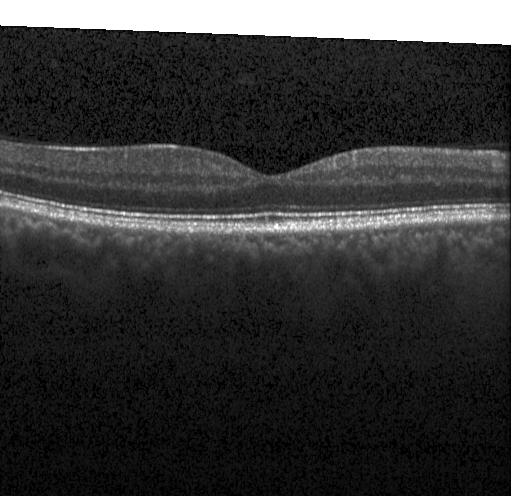
Horizontal scan through the fovea, optical coherence tomography B-scan, acquired on a Heidelberg Spectralis.
Finding: no choroidal neovascularization, no diabetic macular edema, and no drusen.